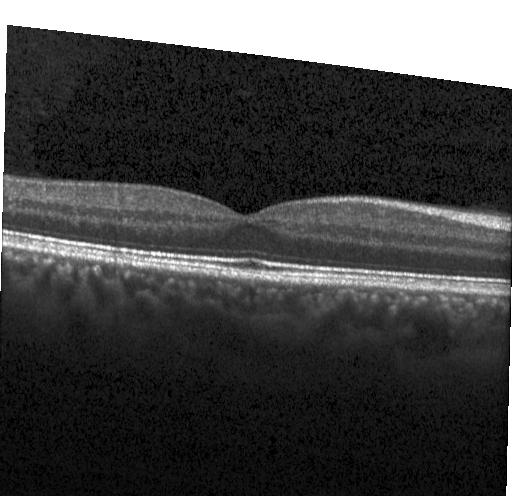
Heidelberg Spectralis OCT system · spectral-domain optical coherence tomography · optical coherence tomography scan.
Assessment: no choroidal neovascularization, diabetic macular edema, or drusen.